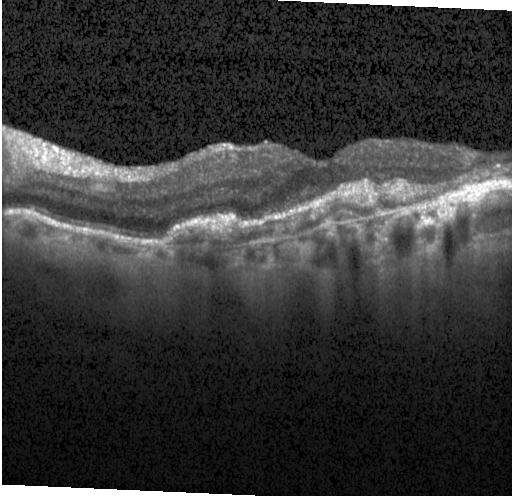

A choroidal neovascular membrane.